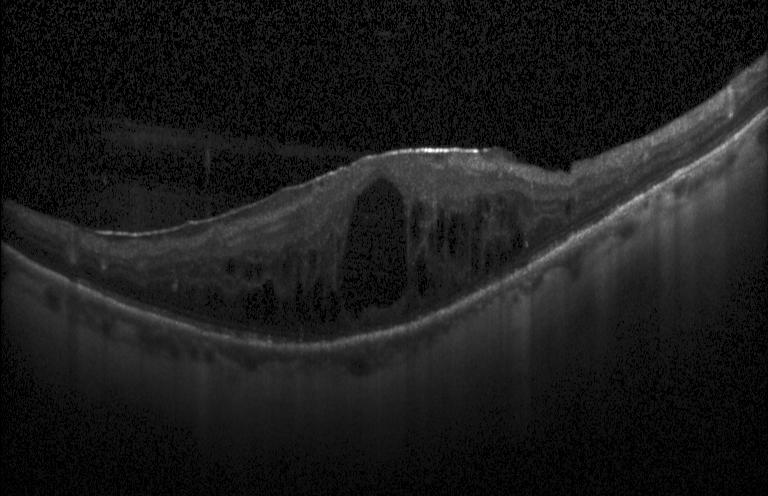 Spectral-domain OCT · retinal OCT cross-section · through the macula · acquired on a Heidelberg Spectralis
Dx: diabetic macular edema (DME).